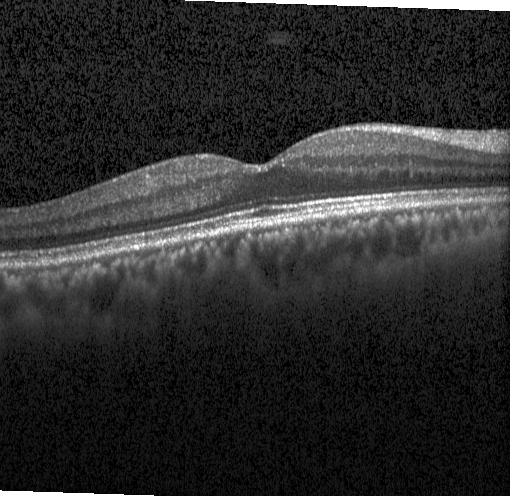

Spectral-domain optical coherence tomography, retinal OCT B-scan. Dx: no choroidal neovascularization, no diabetic macular edema, and no drusen.